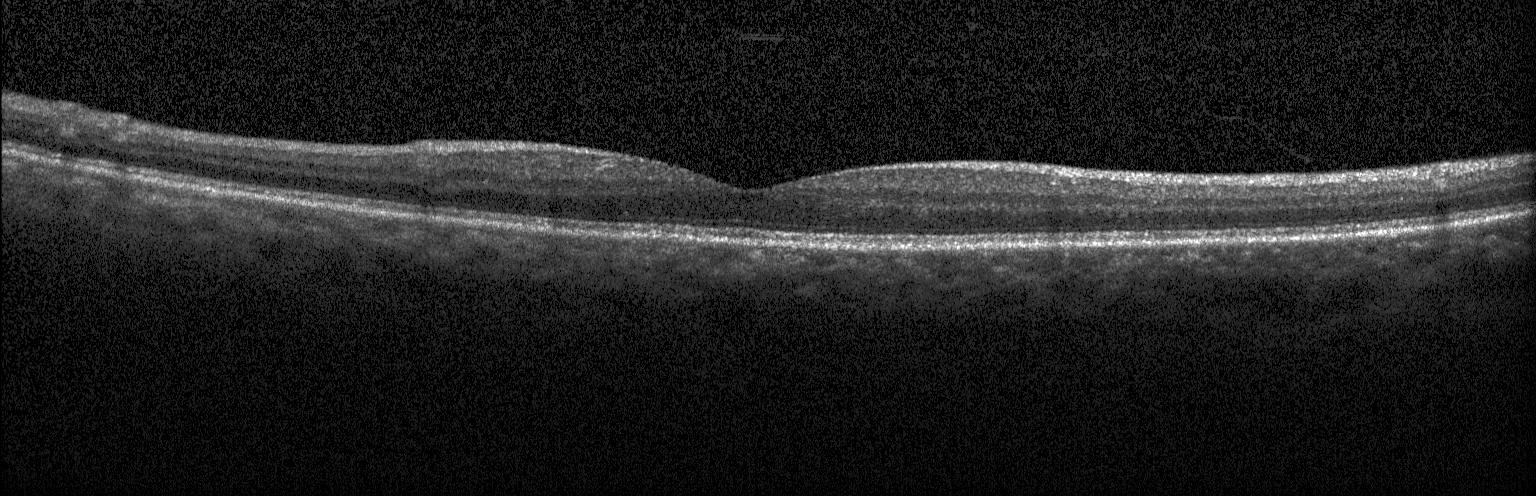

Fovea-centered. Retinal OCT cross-section. SD-OCT.
Assessment: neither choroidal neovascularization, diabetic macular edema, nor drusen.